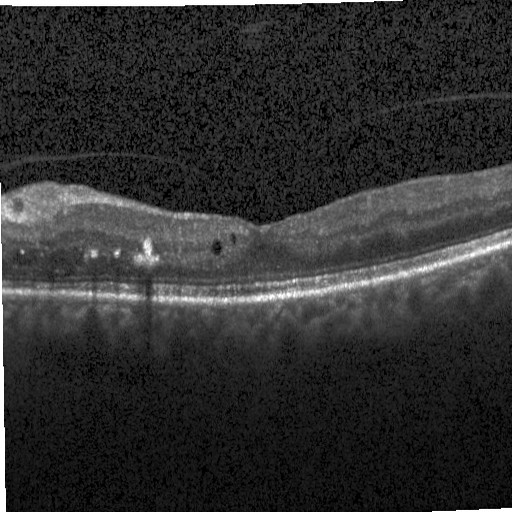

OCT finding: diabetic macular edema.